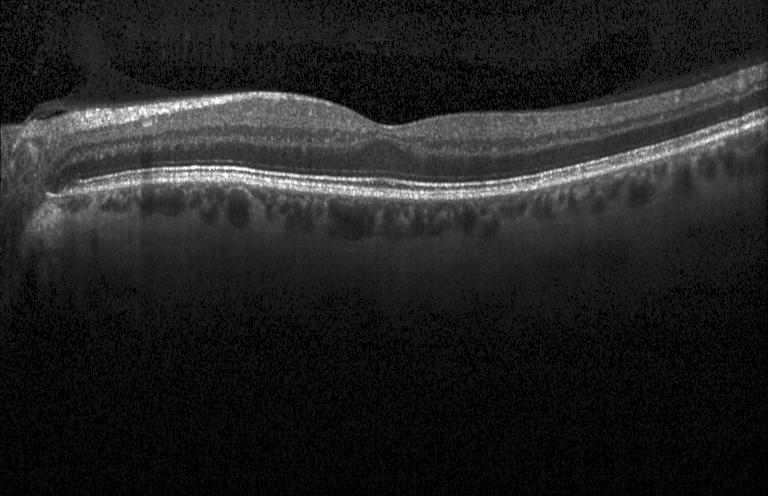
Macular OCT: neither CNV, DME, nor drusen.